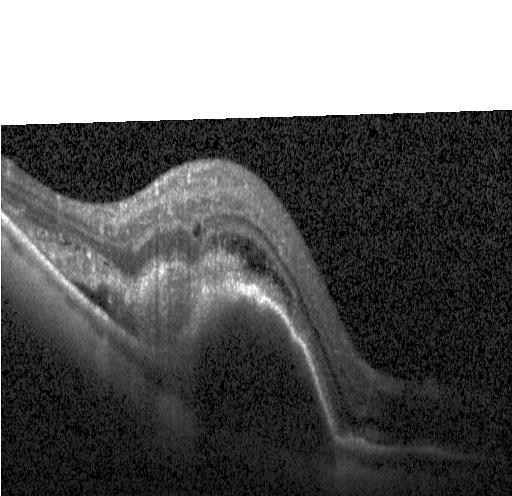 OCT B-scan; through the macula.
Diagnosis: a choroidal neovascular membrane.